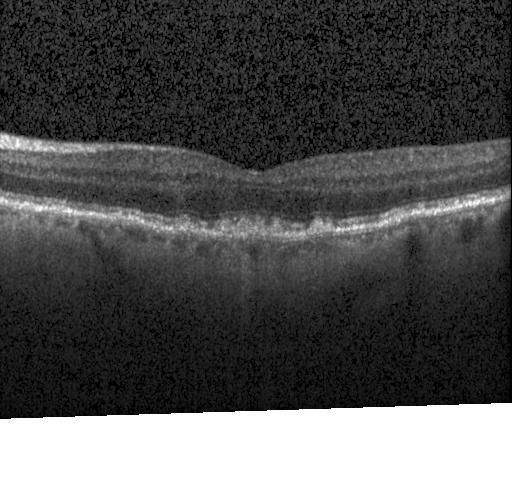 Macular OCT demonstrating drusen.